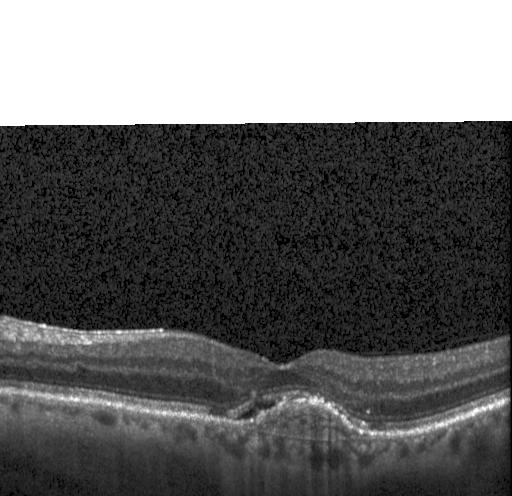

Impression: choroidal neovascularization (CNV).